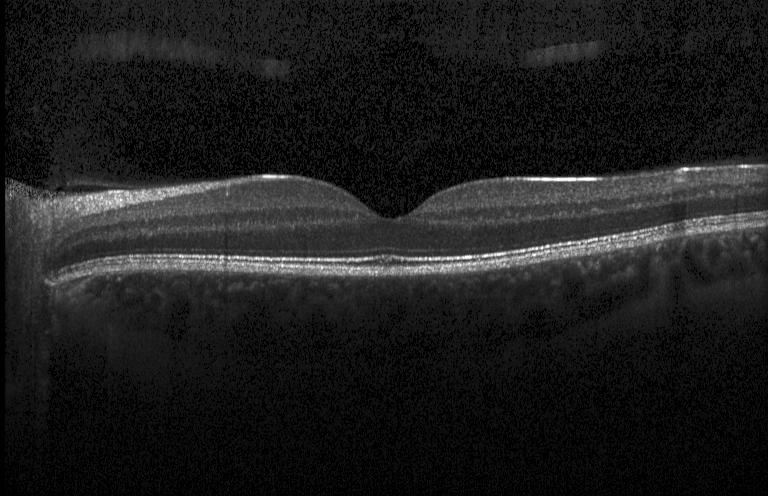 Spectral-domain optical coherence tomography, acquired on a Heidelberg Spectralis, optical coherence tomography B-scan.
Finding: neither choroidal neovascularization, diabetic macular edema, nor drusen.